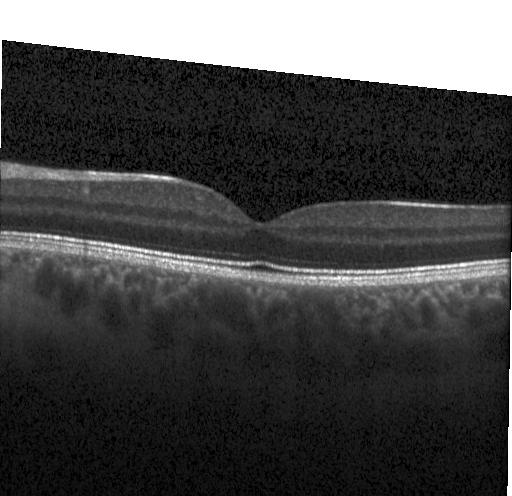 Finding: no evidence of choroidal neovascularization, diabetic macular edema, or drusen.